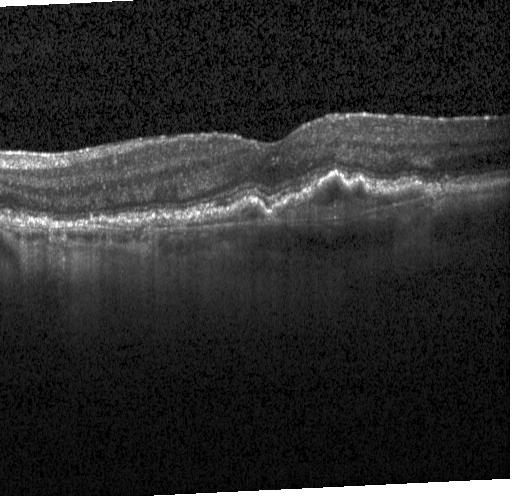

SD-OCT. Optical coherence tomography B-scan. Fovea-centered. A choroidal neovascular membrane.